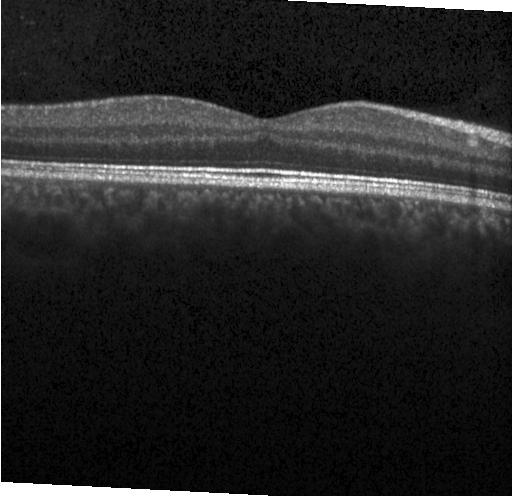
Retinal OCT B-scan. This B-scan demonstrates neither CNV, DME, nor drusen.